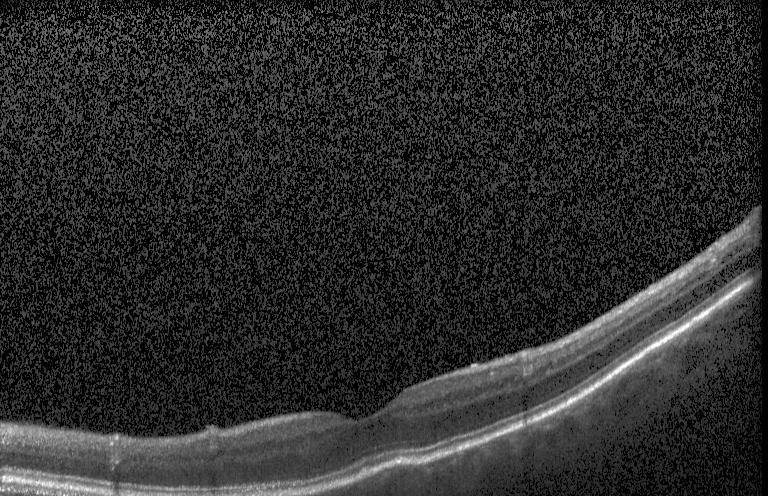

Through the macula. Optical coherence tomography B-scan. Instrument: Heidelberg Spectralis. Spectral-domain optical coherence tomography — Neither choroidal neovascularization, diabetic macular edema, nor drusen.